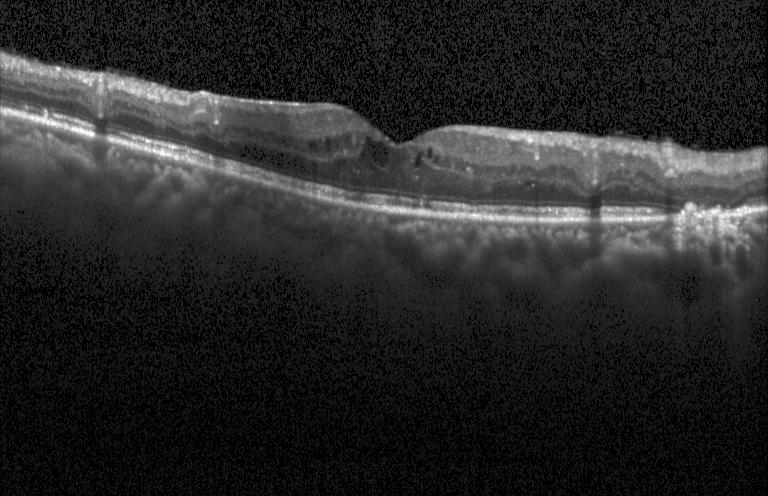 Diagnosis: diabetic macular edema.